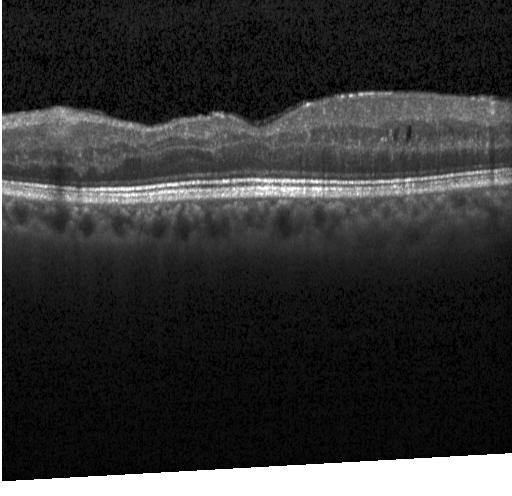
Retinal OCT B-scan, Heidelberg Spectralis — Macular OCT: DME.